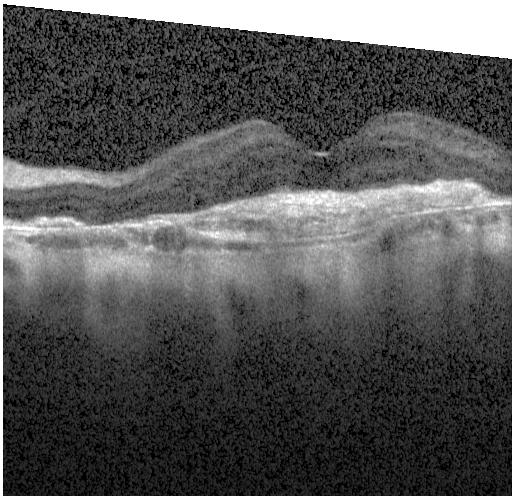 Heidelberg Spectralis OCT system · macular scan · OCT B-scan · SD-OCT.
Dx: a choroidal neovascular membrane.